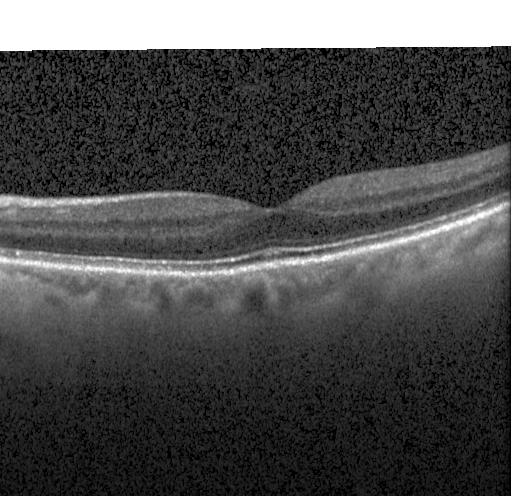
Macular OCT demonstrating neither CNV, DME, nor drusen.